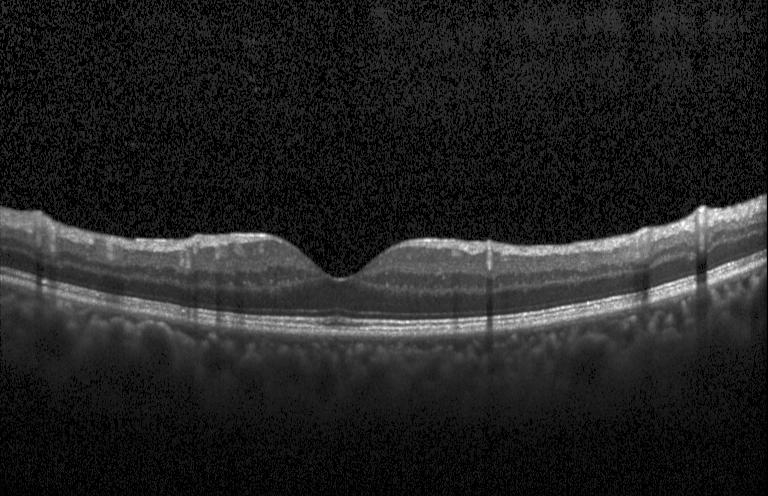
This B-scan demonstrates neither choroidal neovascularization, diabetic macular edema, nor drusen.